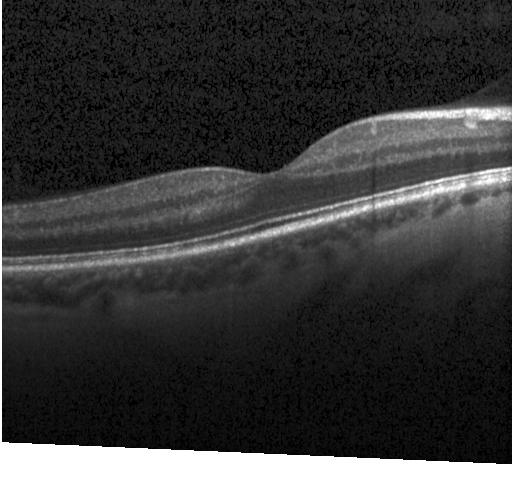 Retinal OCT cross-section · spectral-domain OCT.
The scan shows neither CNV, DME, nor drusen.